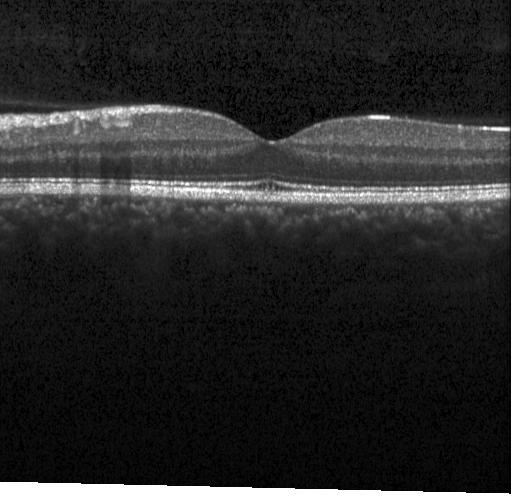
Retinal OCT cross-section showing no choroidal neovascularization, diabetic macular edema, or drusen.